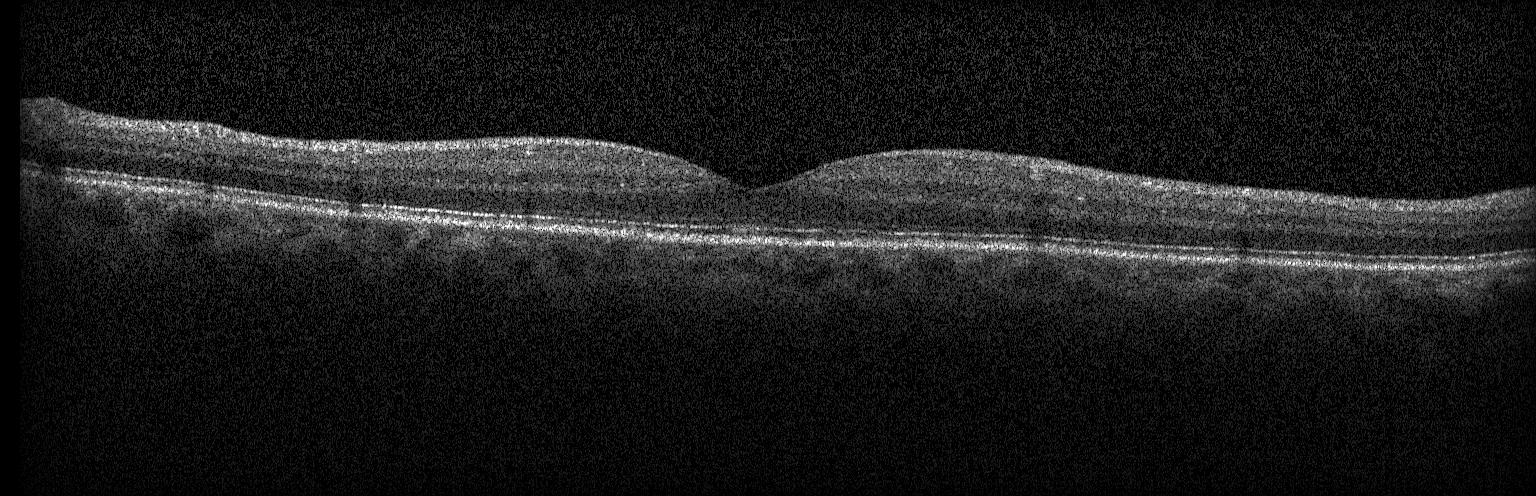 Dx: neither choroidal neovascularization, diabetic macular edema, nor drusen.